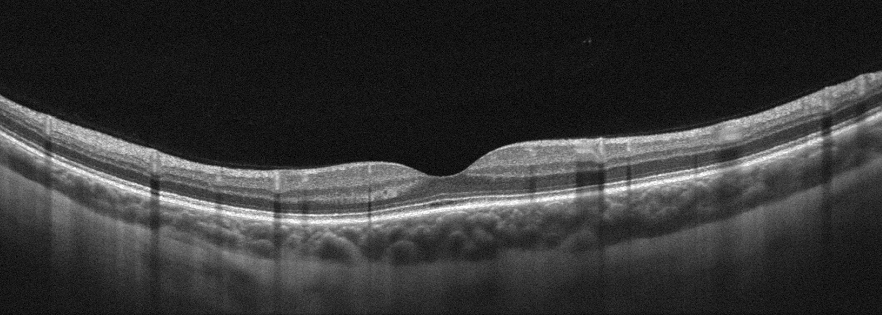 Through the macula, Optovue Avanti RTVue XR, retinal OCT cross-section, OD. The scan shows no evidence of AMD, DME, ERM, RAO, RVO, or VID.